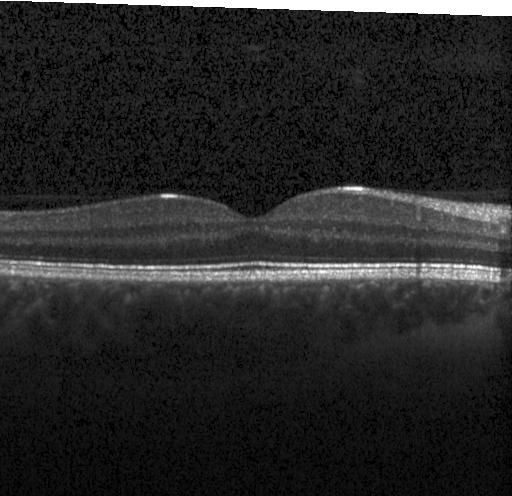 Retinal OCT cross-section
Finding: no evidence of choroidal neovascularization, diabetic macular edema, or drusen.